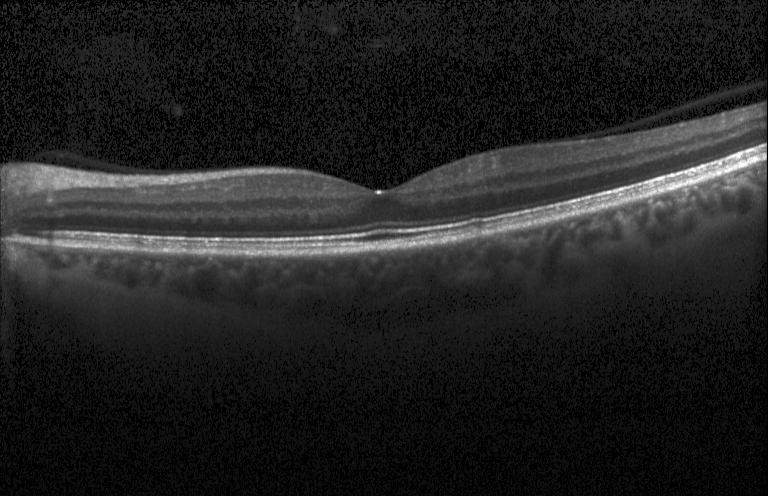
Retinal OCT B-scan, instrument: Heidelberg Spectralis — Impression: neither choroidal neovascularization, diabetic macular edema, nor drusen.